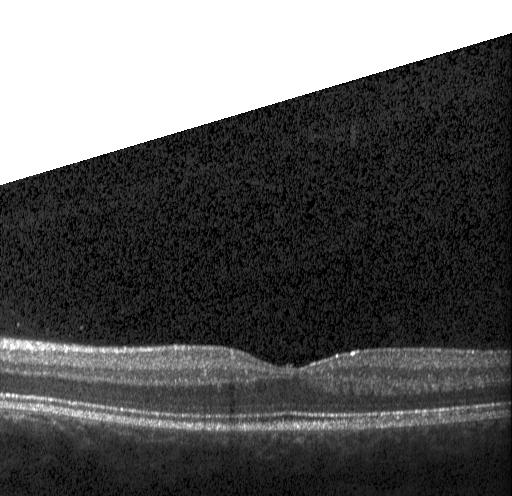 Retinal OCT B-scan.
Diagnosis: no choroidal neovascularization, no diabetic macular edema, and no drusen.